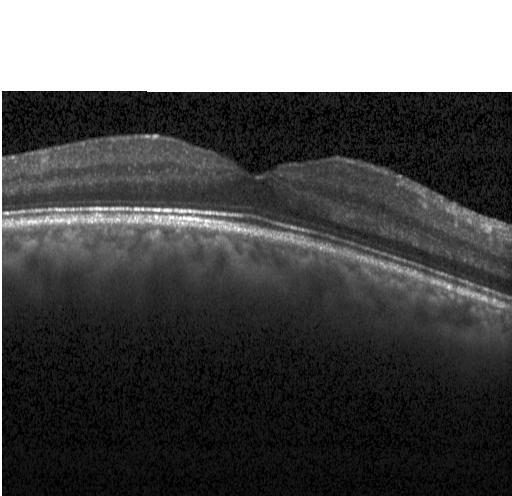 Optical coherence tomography B-scan; SD-OCT; Heidelberg Spectralis OCT system.
Macular OCT: no choroidal neovascularization, diabetic macular edema, or drusen.